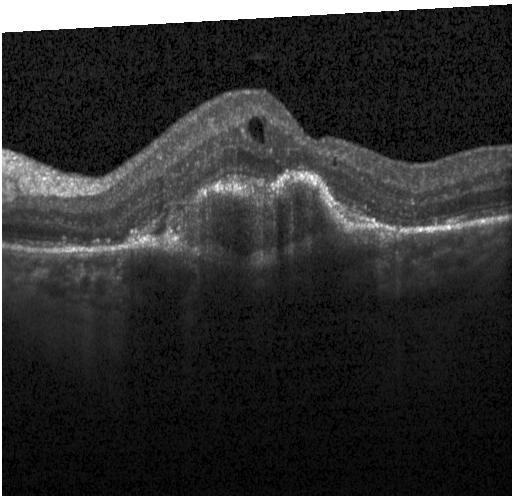
The scan shows a choroidal neovascular membrane.